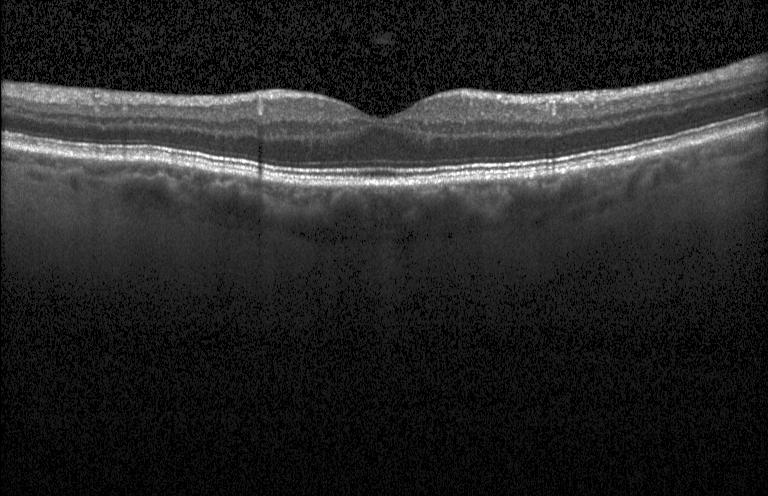

OCT line scan.
The scan shows neither choroidal neovascularization, diabetic macular edema, nor drusen.